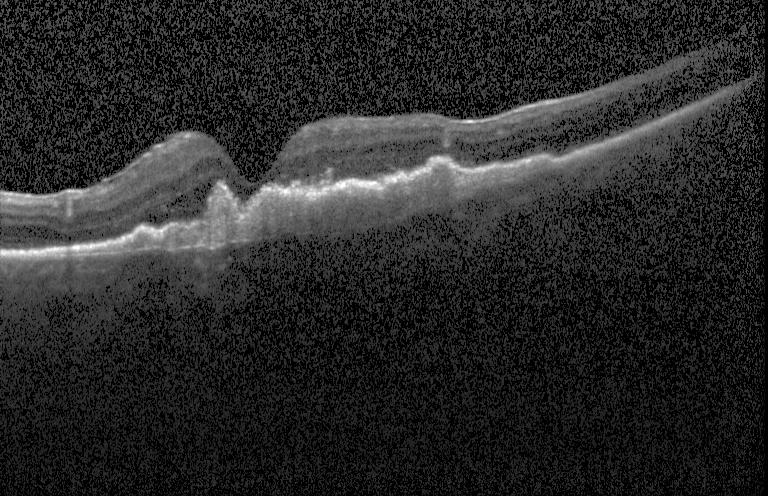 Optical coherence tomography B-scan; macular scan; Heidelberg Spectralis.
Choroidal neovascularization (CNV).